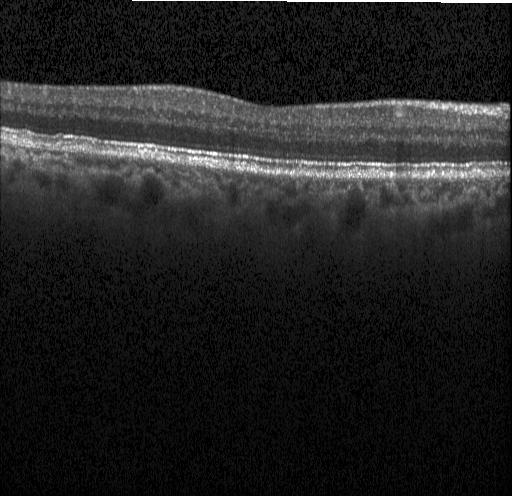

OCT B-scan.
Impression: no choroidal neovascularization, no diabetic macular edema, and no drusen.